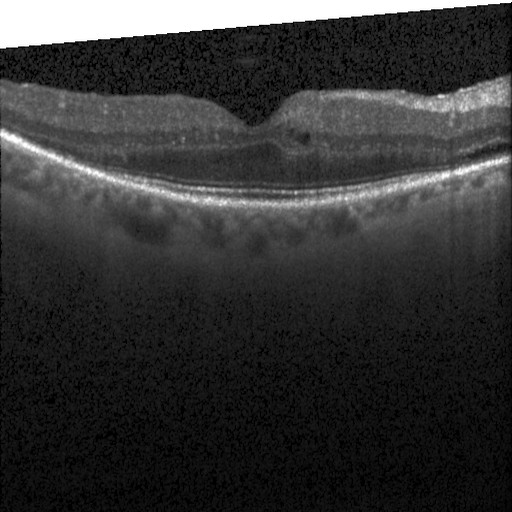

Impression: diabetic macular edema.